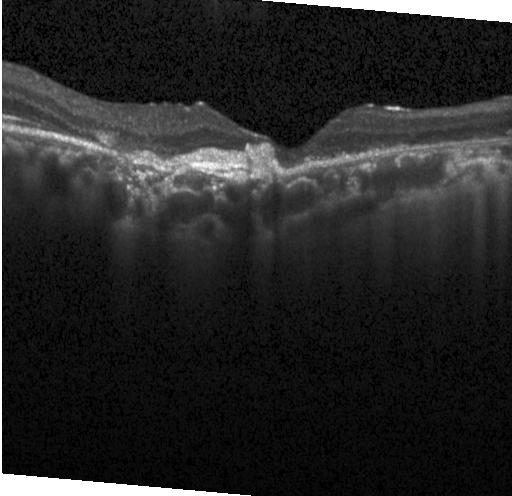

Diagnosis: a choroidal neovascular membrane.